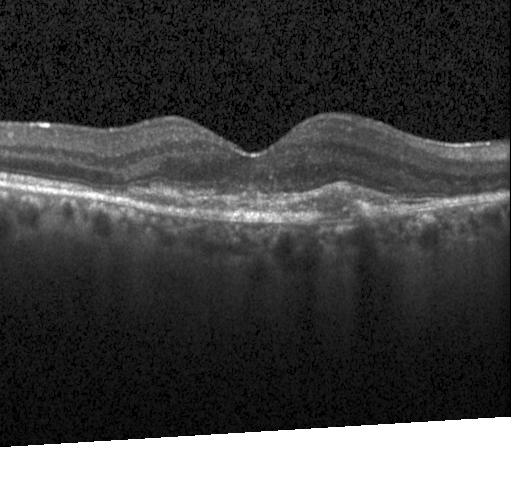 Macular scan, OCT line scan, SD-OCT — Finding: choroidal neovascularization.